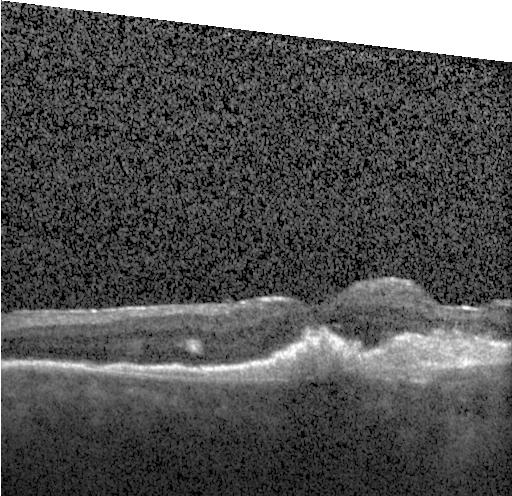

Finding: choroidal neovascularization.